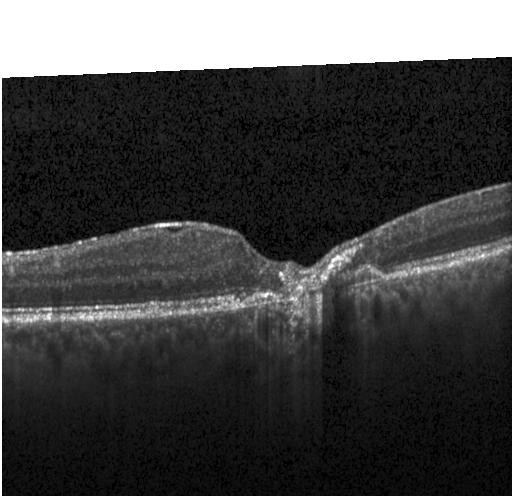

Macular OCT: CNV.